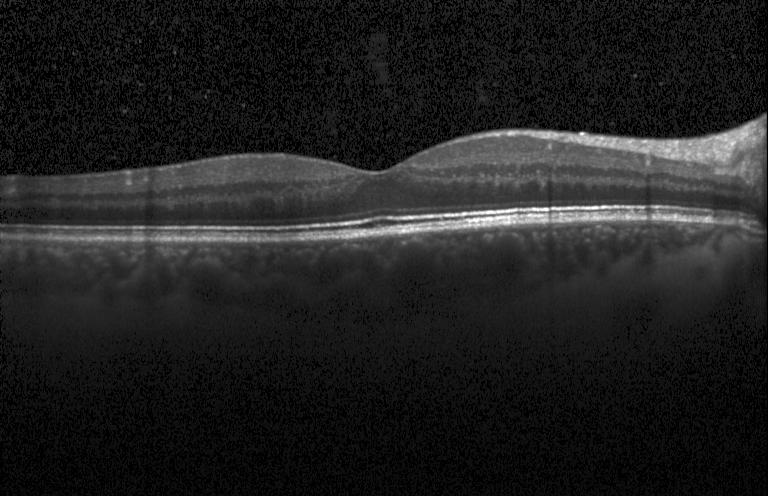

OCT finding: no CNV, DME, or drusen.